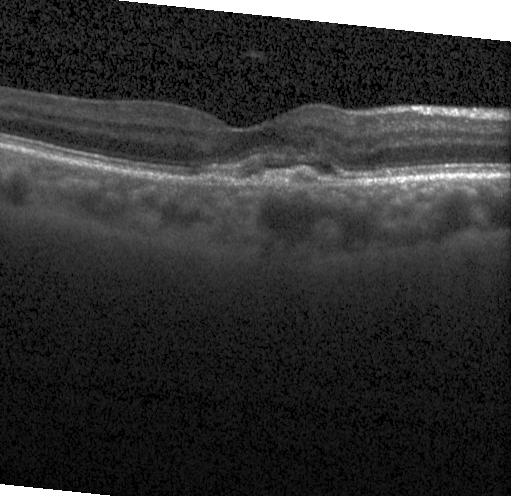
OCT line scan
Choroidal neovascularization.